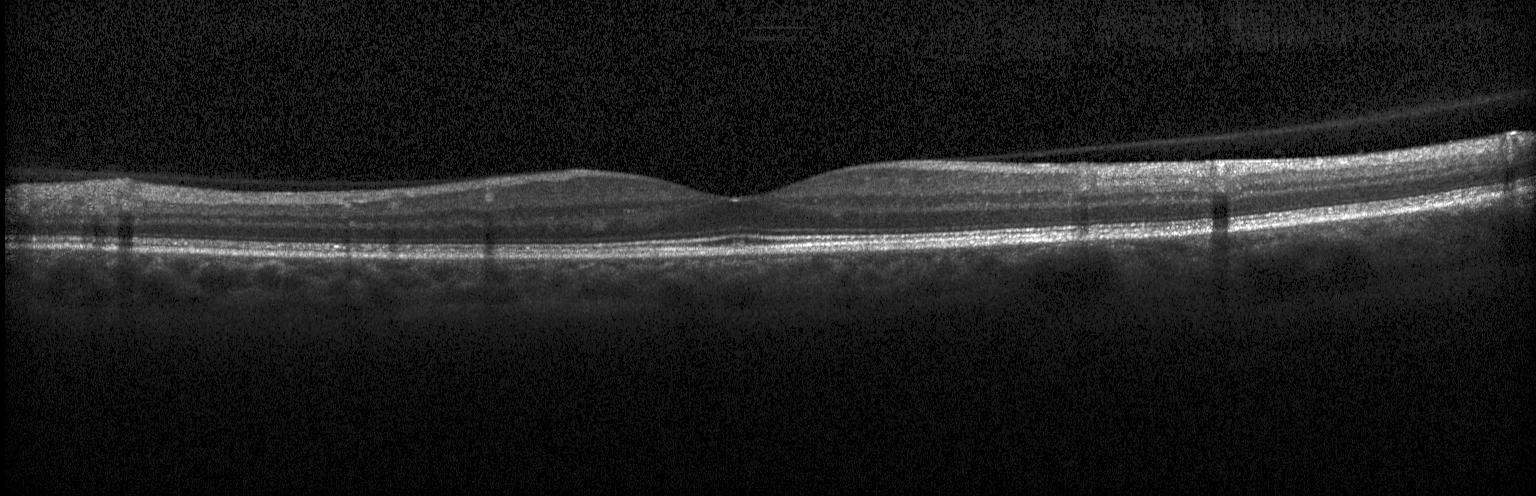 Horizontal scan through the fovea. OCT B-scan. SD-OCT — The scan shows no evidence of choroidal neovascularization, diabetic macular edema, or drusen.